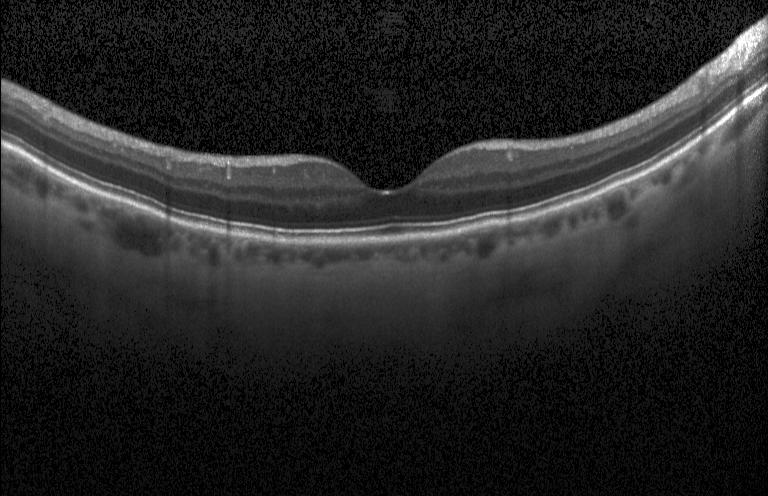
Assessment: no evidence of choroidal neovascularization, diabetic macular edema, or drusen.